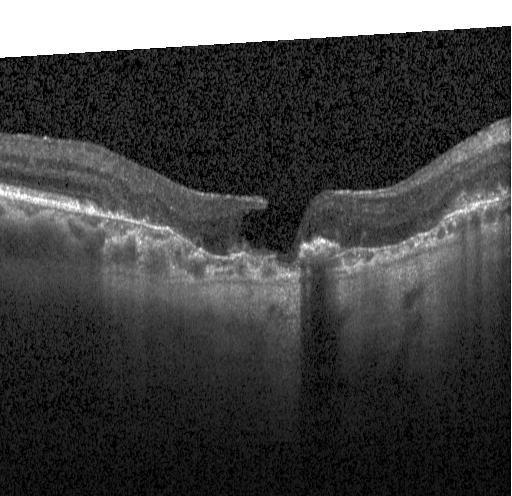

Spectral-domain OCT · fovea-centered · OCT line scan
The scan shows choroidal neovascularization.